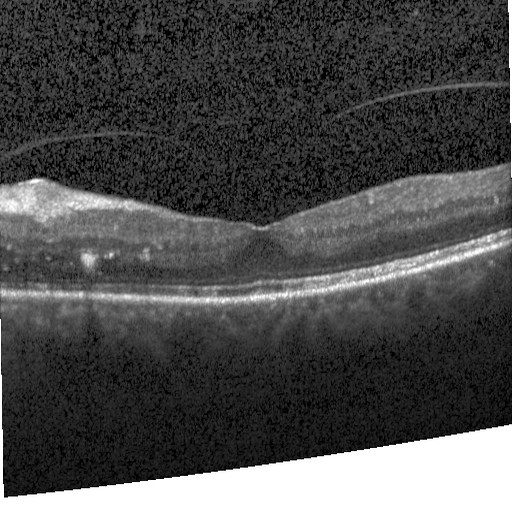
Macular OCT: DME.